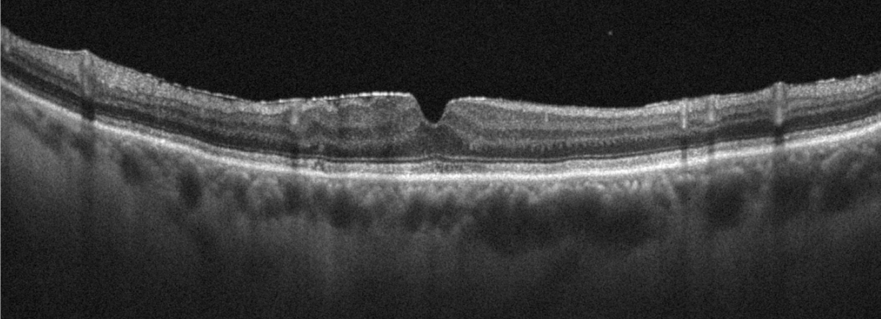
Finding: ERM.